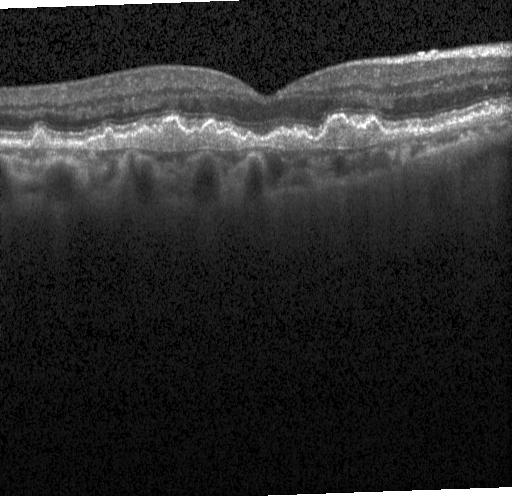

Acquired on a Heidelberg Spectralis; retinal OCT cross-section
This B-scan demonstrates a choroidal neovascular membrane.